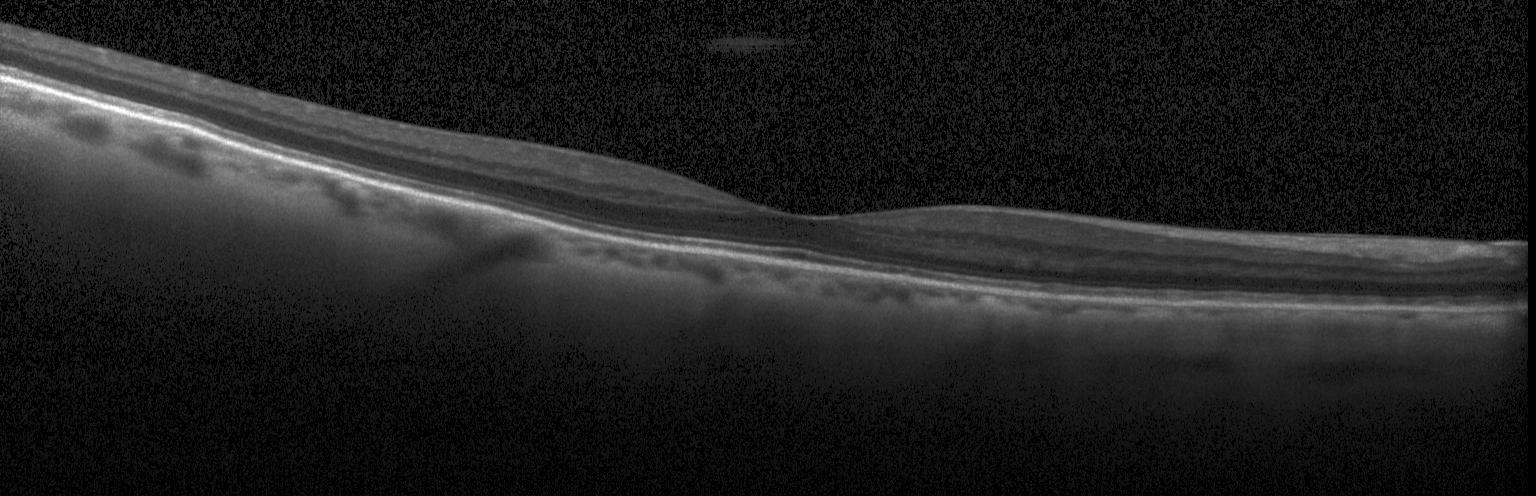

OCT scan showing neither choroidal neovascularization, diabetic macular edema, nor drusen.